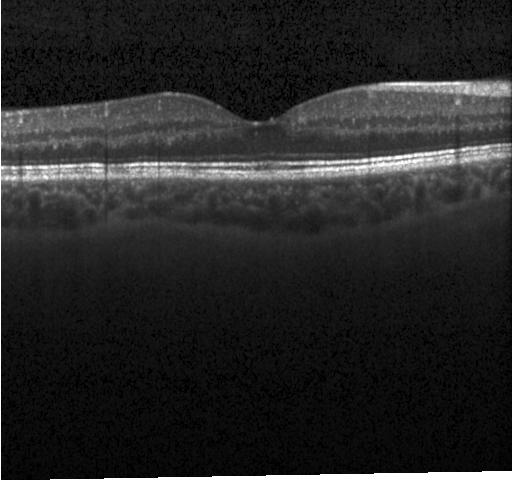 Impression: no CNV, DME, or drusen.